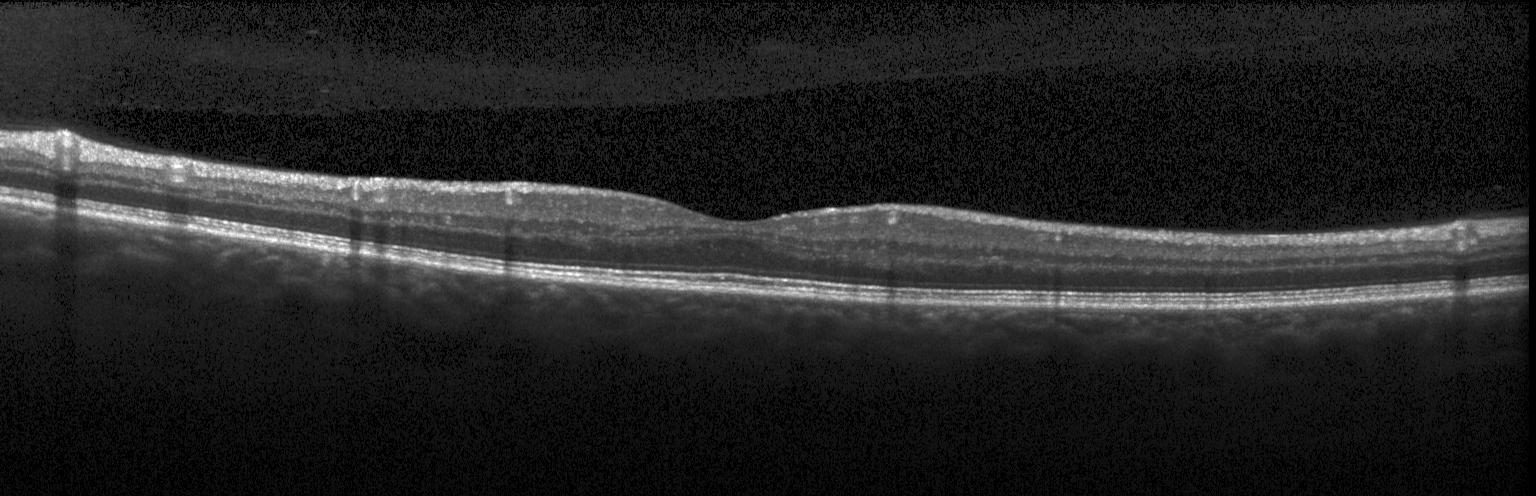 Finding: no evidence of CNV, DME, or drusen.